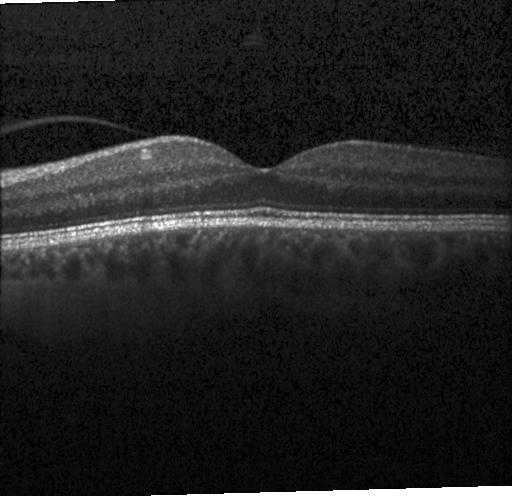

Optical coherence tomography scan. Heidelberg Spectralis OCT system. Spectral-domain optical coherence tomography. The scan shows no evidence of CNV, DME, or drusen.